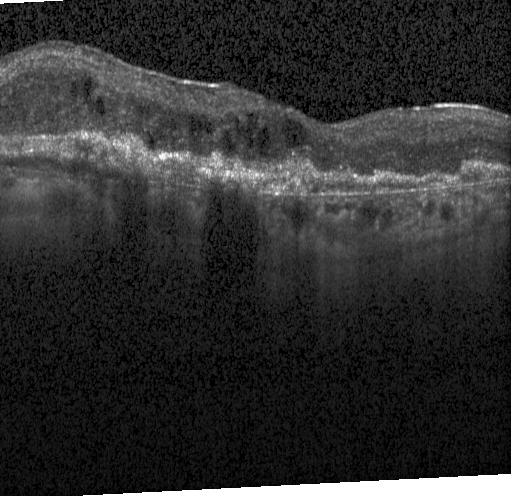
OCT B-scan. Finding: a choroidal neovascular membrane.